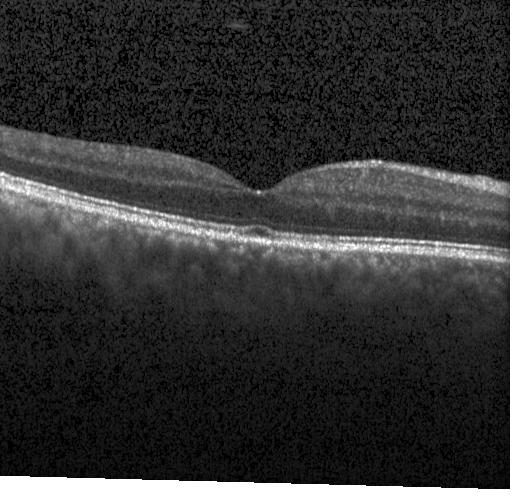 Spectral-domain optical coherence tomography; Heidelberg Spectralis OCT system; optical coherence tomography scan. Assessment: no choroidal neovascularization, no diabetic macular edema, and no drusen.